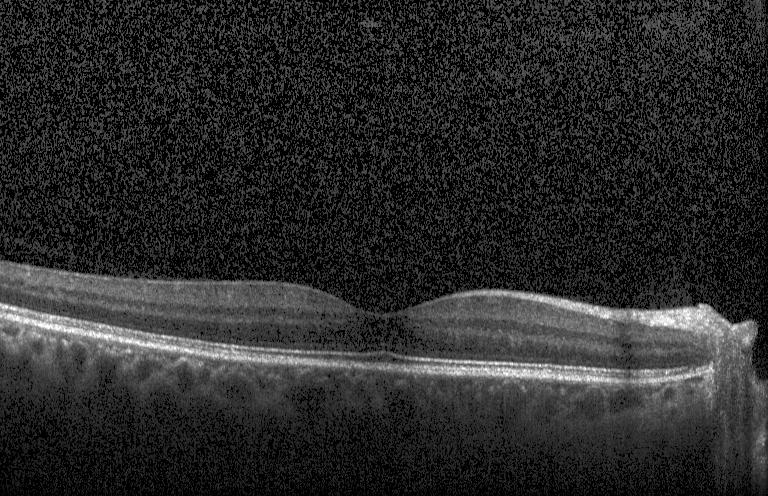
Diagnosis: no choroidal neovascularization, diabetic macular edema, or drusen.